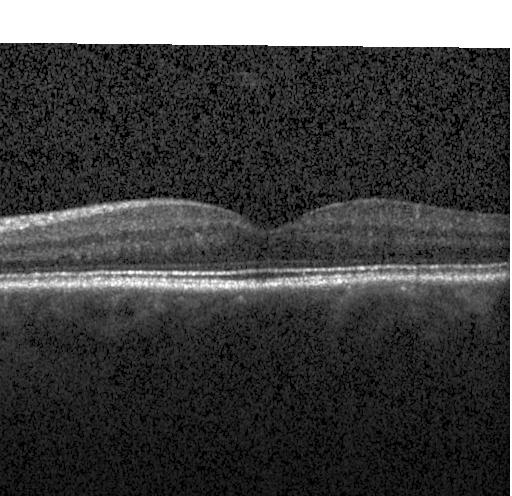 OCT line scan; horizontal scan through the fovea; acquired on a Heidelberg Spectralis; spectral-domain optical coherence tomography.
Assessment: no evidence of CNV, DME, or drusen.